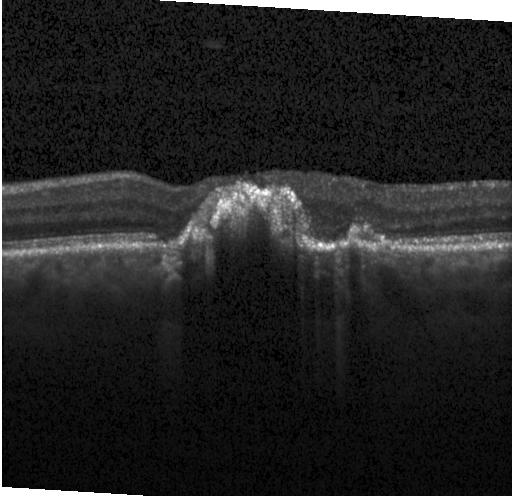
Retinal OCT cross-section showing choroidal neovascularization.